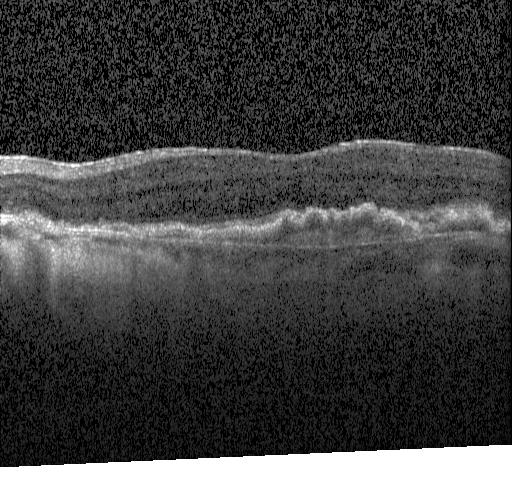 Retinal OCT cross-section · Heidelberg Spectralis · SD-OCT · centered on the fovea — Assessment: a choroidal neovascular membrane.